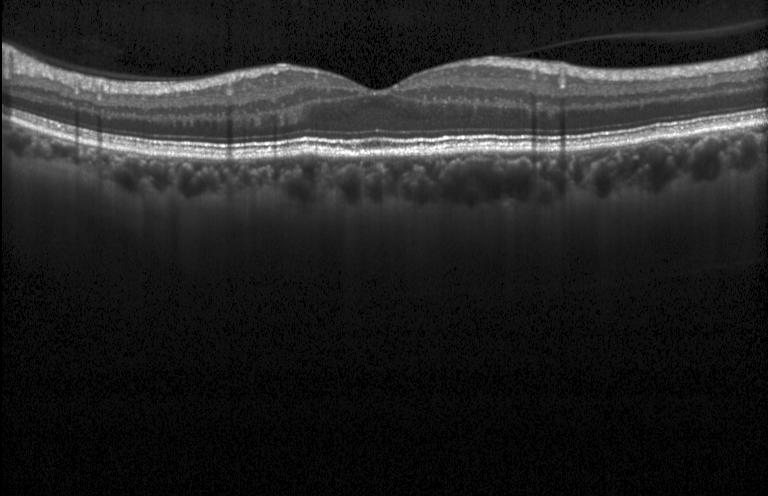 Diagnosis: no choroidal neovascularization, diabetic macular edema, or drusen.